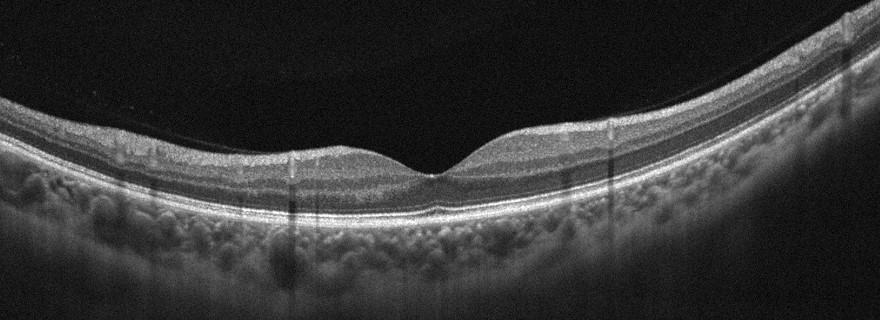 Macular OCT demonstrating absence of AMD, DME, ERM, RAO, RVO, and vitreomacular interface disease.